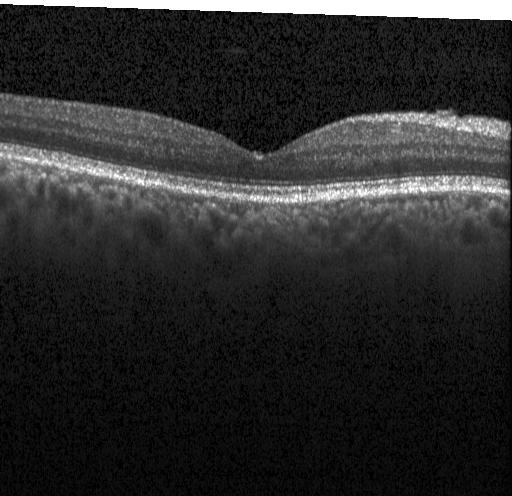
OCT B-scan, spectral-domain OCT — Macular OCT: no evidence of CNV, DME, or drusen.